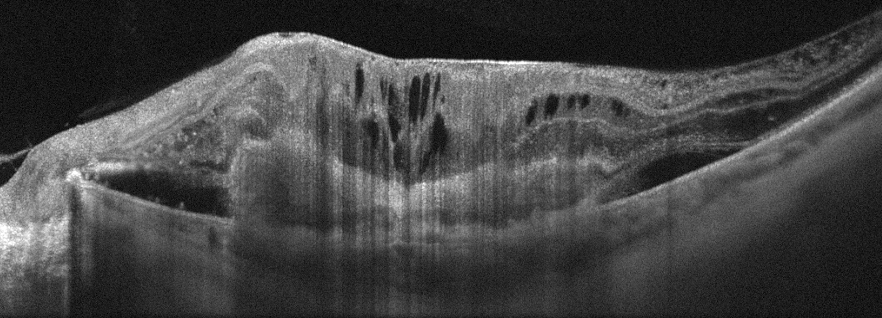
Optical coherence tomography B-scan.
Dx: AMD.